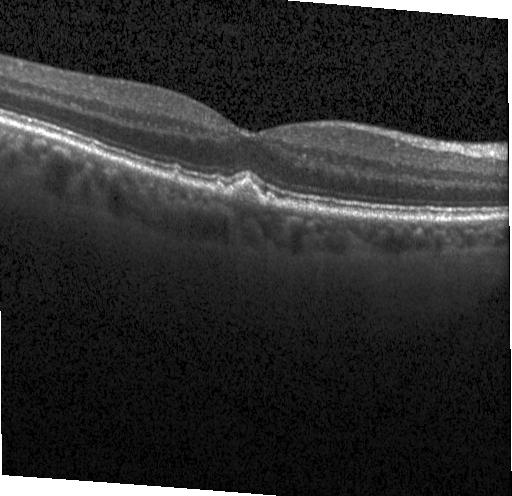

Assessment: drusen.